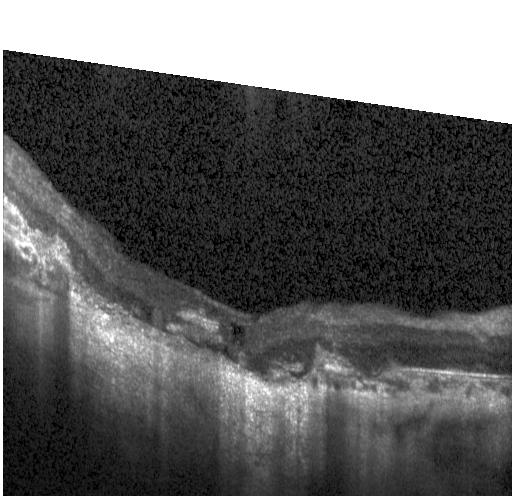
The scan shows a choroidal neovascular membrane.